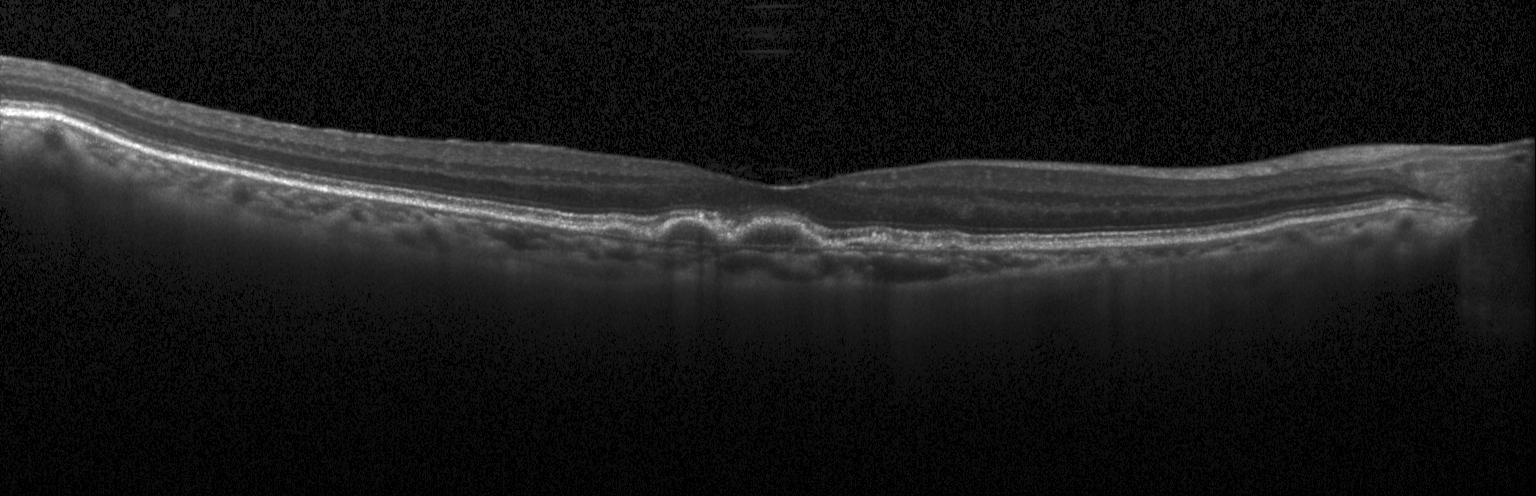
Spectral-domain OCT B-scan: CNV.